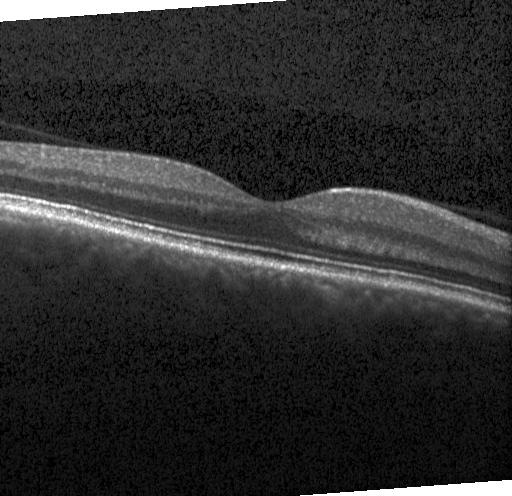
OCT finding: neither choroidal neovascularization, diabetic macular edema, nor drusen.